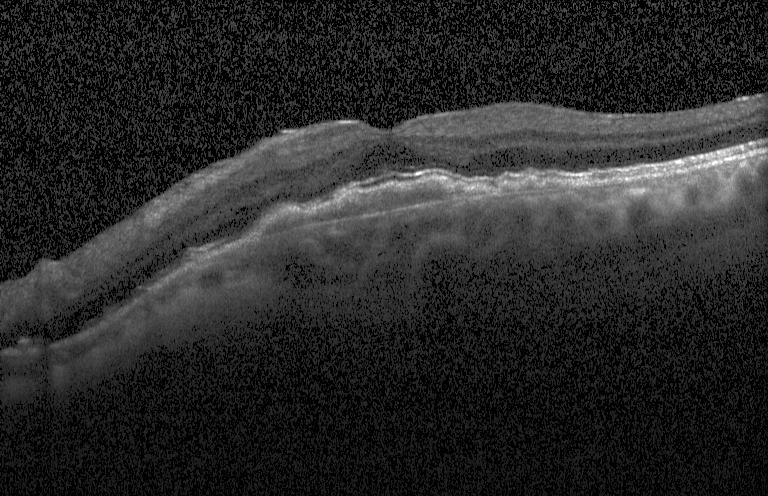 Retinal OCT cross-section. Macular scan.
Finding: a choroidal neovascular membrane.